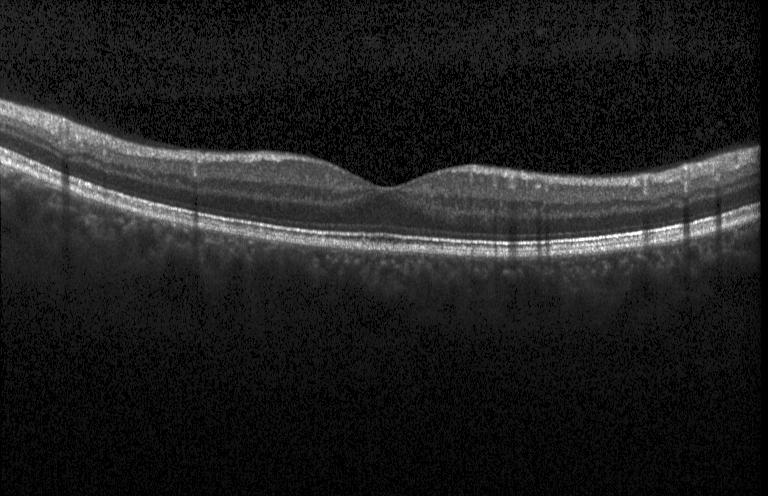 Optical coherence tomography scan. Impression: neither choroidal neovascularization, diabetic macular edema, nor drusen.